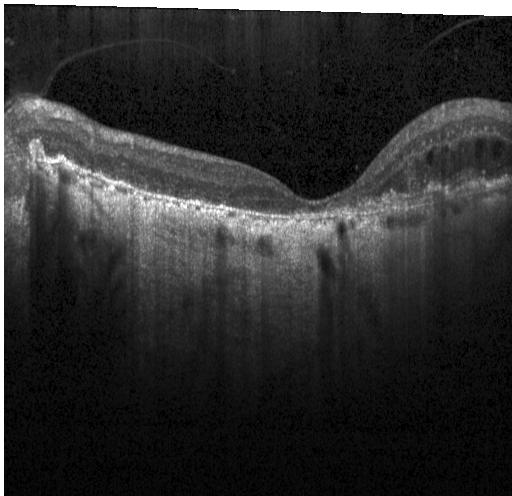

SD-OCT; retinal OCT B-scan.
Dx: choroidal neovascularization.